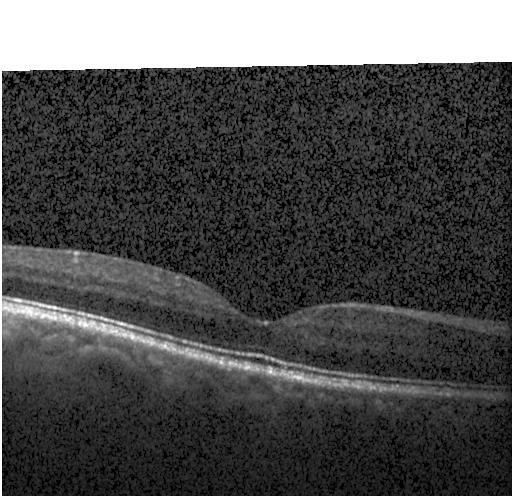
Spectral-domain optical coherence tomography, optical coherence tomography B-scan.
Diagnosis: no evidence of choroidal neovascularization, diabetic macular edema, or drusen.